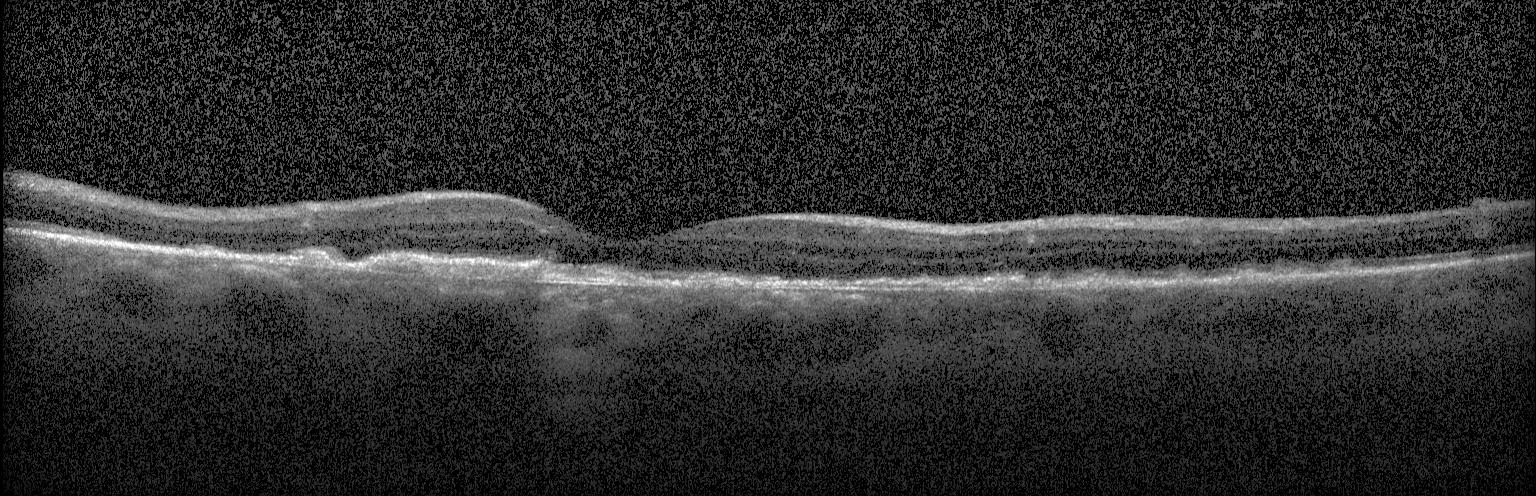

OCT B-scan.
Assessment: CNV.